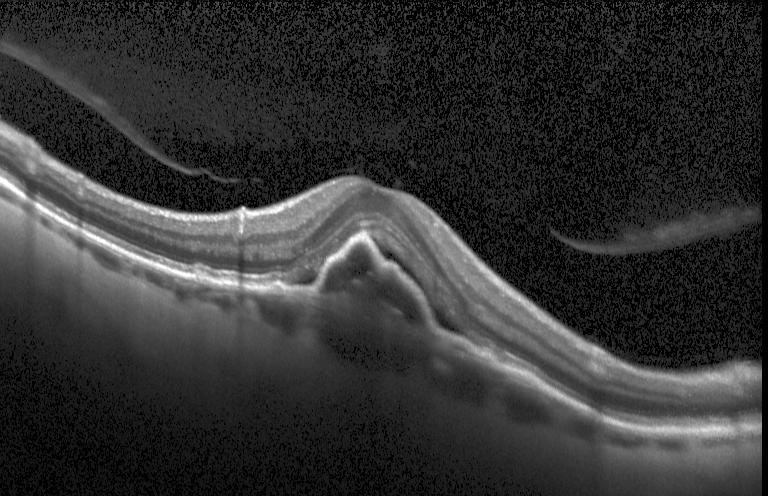

Assessment: choroidal neovascularization (CNV).